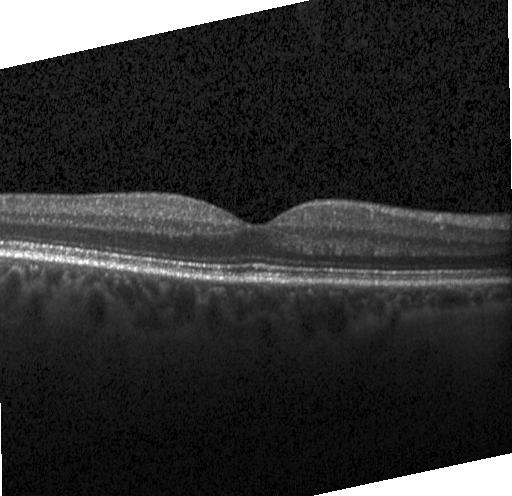

Diagnosis: neither choroidal neovascularization, diabetic macular edema, nor drusen.